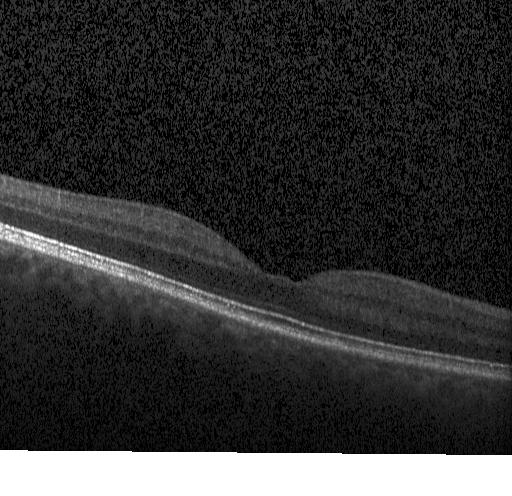
Optical coherence tomography scan; spectral-domain optical coherence tomography; macular scan
Impression: no choroidal neovascularization, no diabetic macular edema, and no drusen.